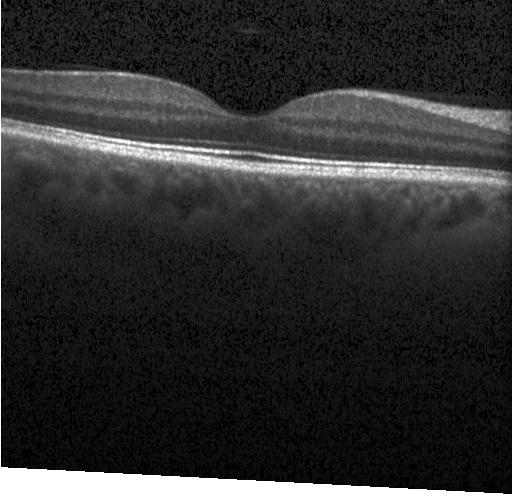

Finding: neither choroidal neovascularization, diabetic macular edema, nor drusen.